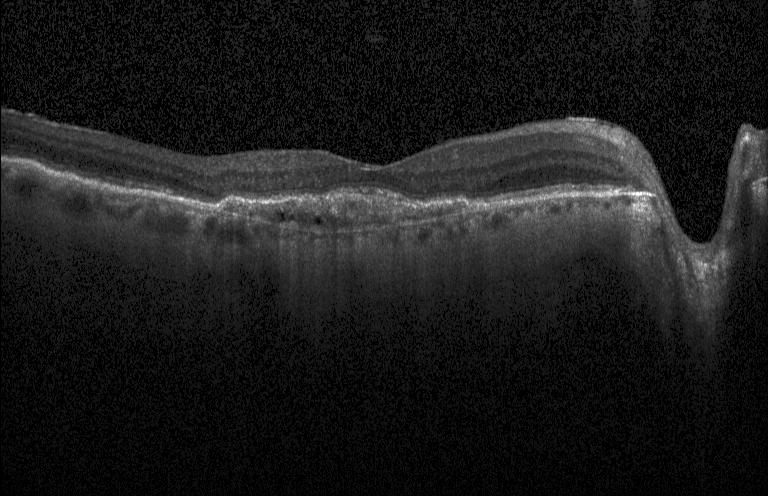

Acquired on a Heidelberg Spectralis; retinal OCT cross-section
This B-scan demonstrates choroidal neovascularization (CNV).